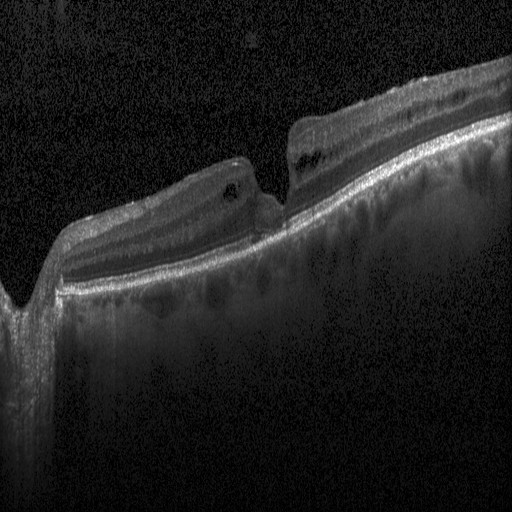
Heidelberg Spectralis OCT system; horizontal scan through the fovea; OCT line scan — Assessment: DME.